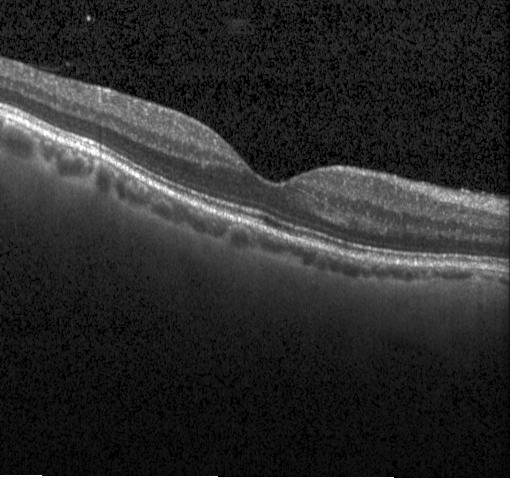

Optical coherence tomography B-scan — Diagnosis: no choroidal neovascularization, diabetic macular edema, or drusen.